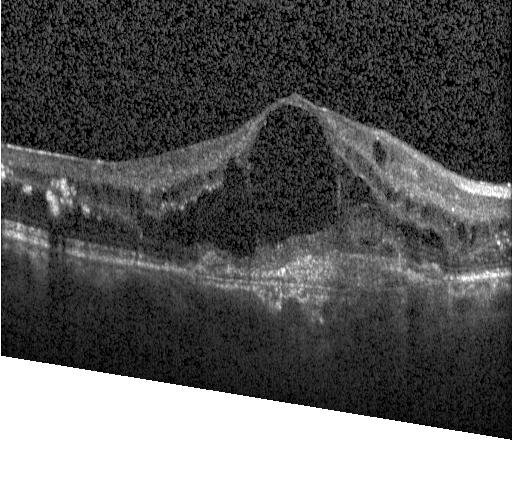

OCT scan showing a choroidal neovascular membrane.